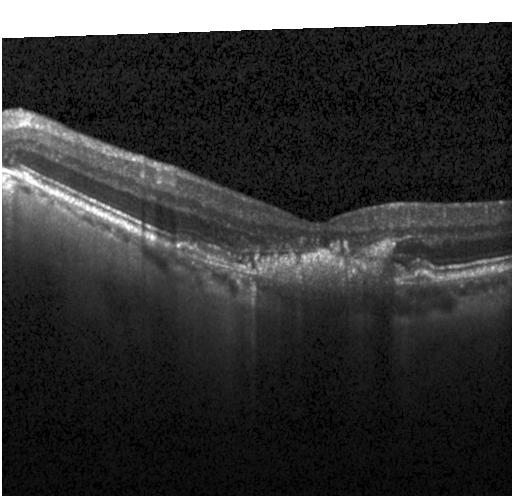
Instrument: Heidelberg Spectralis. Spectral-domain optical coherence tomography. Retinal OCT cross-section. Horizontal scan through the fovea.
The scan shows choroidal neovascularization.